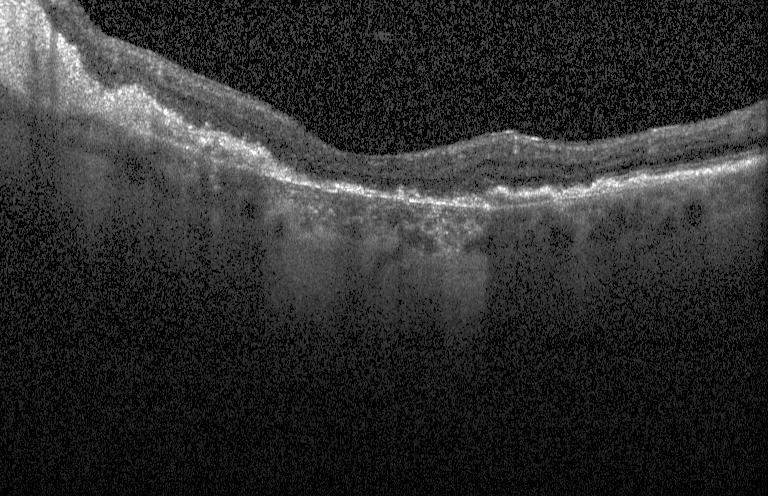

Acquired on a Heidelberg Spectralis. Through the macula. Spectral-domain OCT. Optical coherence tomography B-scan.
Impression: CNV.